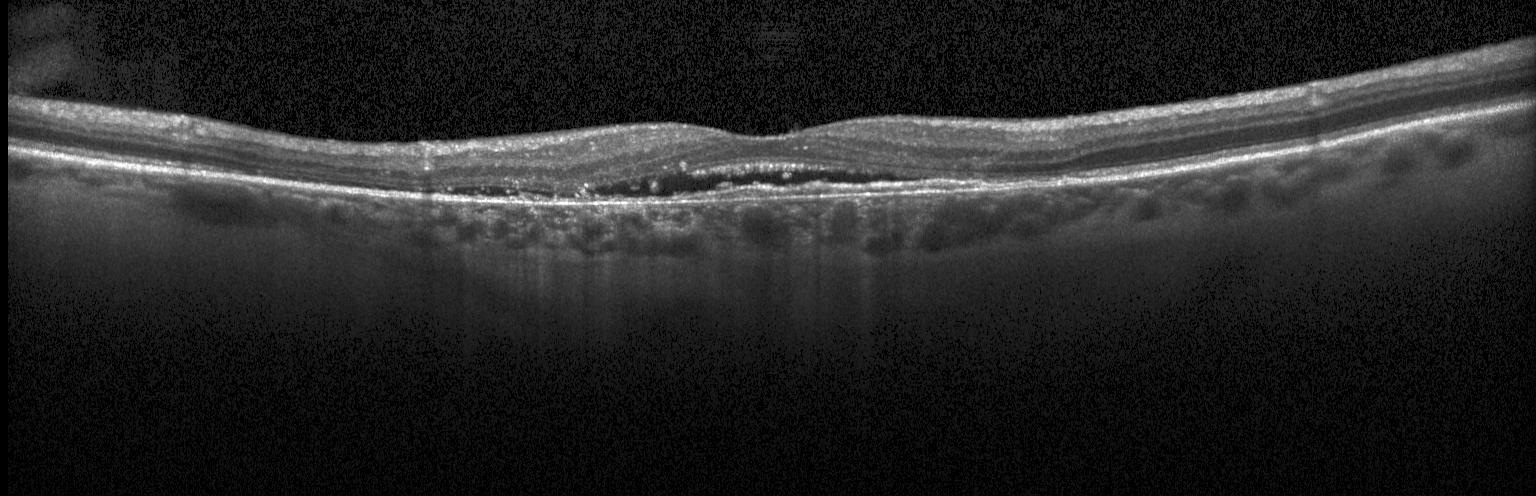 Retinal OCT B-scan, fovea-centered. This B-scan demonstrates CNV.